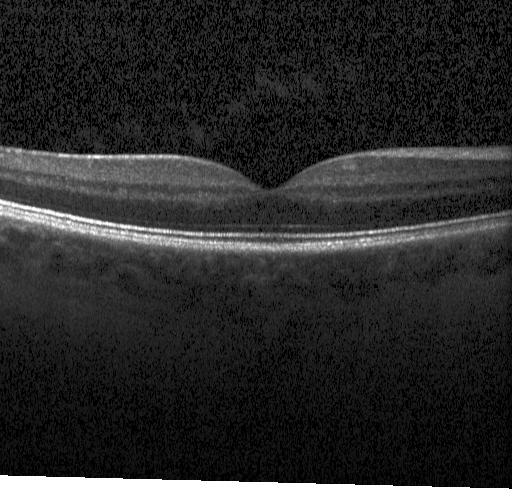 Retinal OCT cross-section. Finding: no choroidal neovascularization, diabetic macular edema, or drusen.